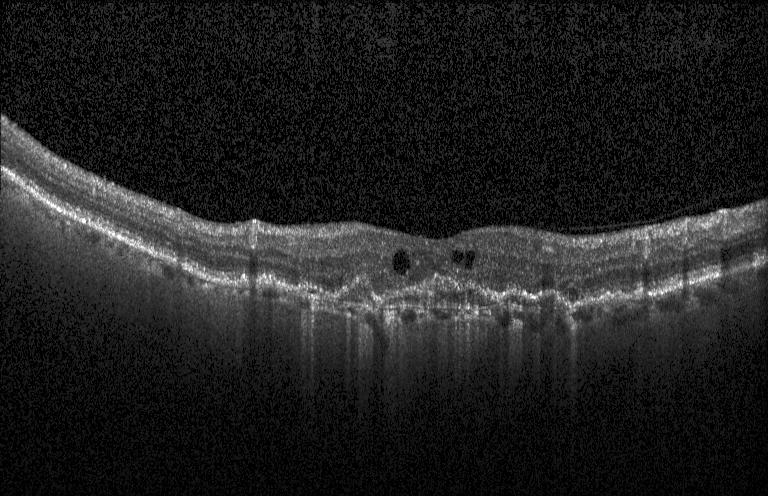

Retinal OCT cross-section
Assessment: a choroidal neovascular membrane.